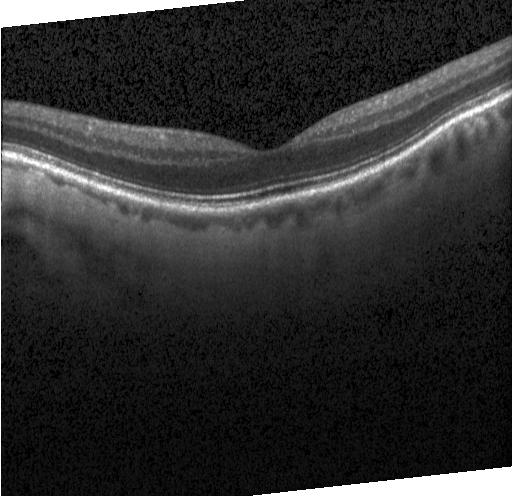

Retinal OCT cross-section. Spectral-domain OCT. Heidelberg Spectralis. Through the macula
Diagnosis: no choroidal neovascularization, no diabetic macular edema, and no drusen.